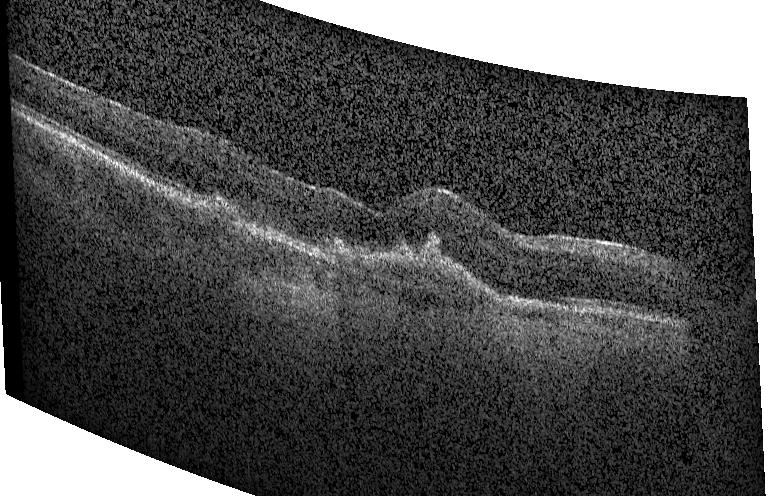
OCT line scan
Finding: CNV.